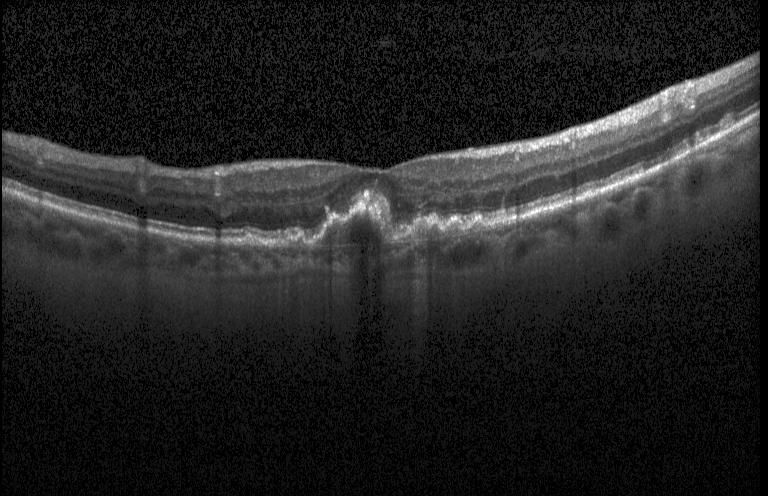
Retinal OCT cross-section · macular scan · spectral-domain optical coherence tomography. This B-scan demonstrates a choroidal neovascular membrane.